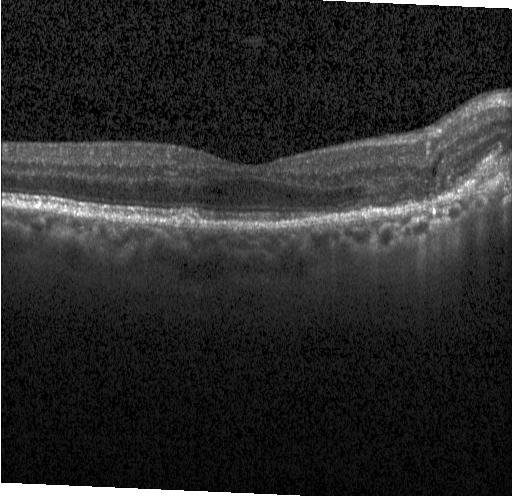
Macular scan; spectral-domain optical coherence tomography; OCT B-scan; acquired on a Heidelberg Spectralis — Diagnosis: a choroidal neovascular membrane.